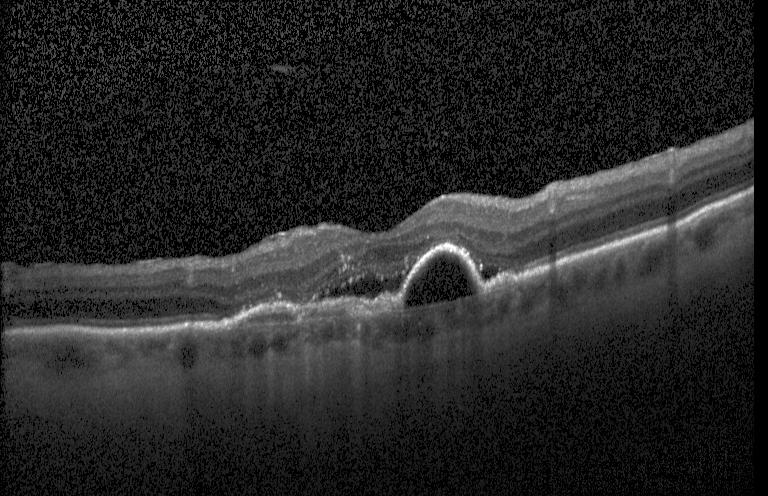

OCT finding: a choroidal neovascular membrane.